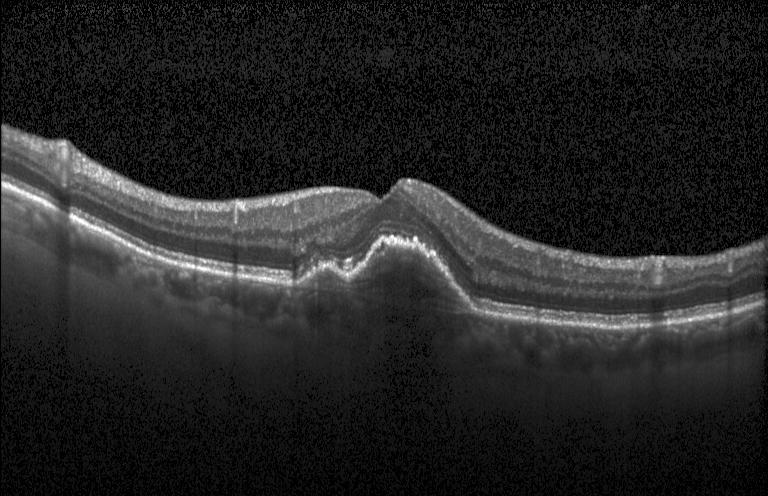
Dx: choroidal neovascularization.